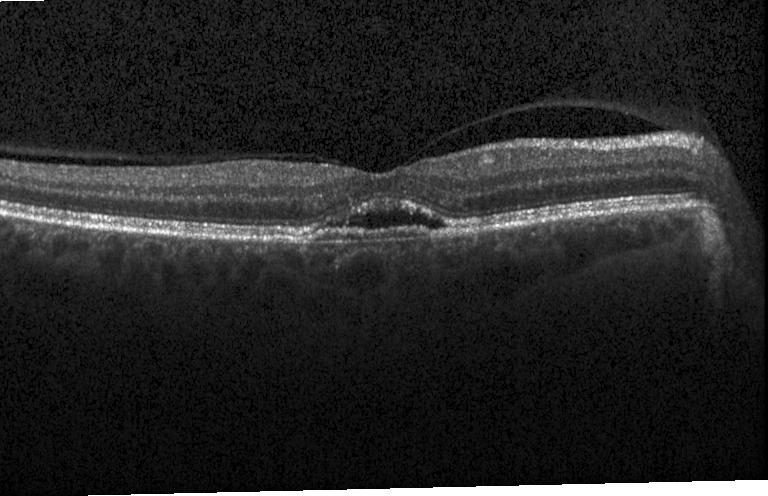
Retinal OCT cross-section showing a choroidal neovascular membrane.